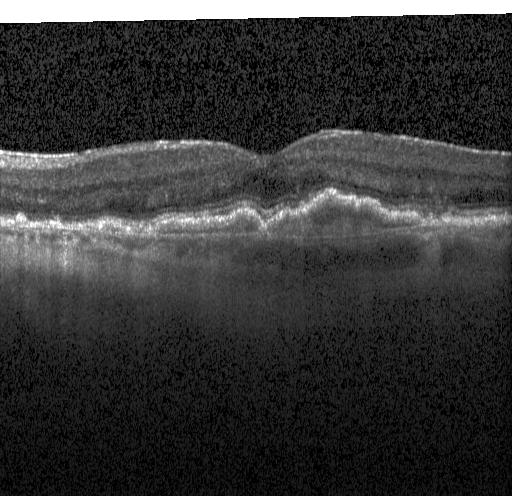
Optical coherence tomography B-scan. Finding: a choroidal neovascular membrane.